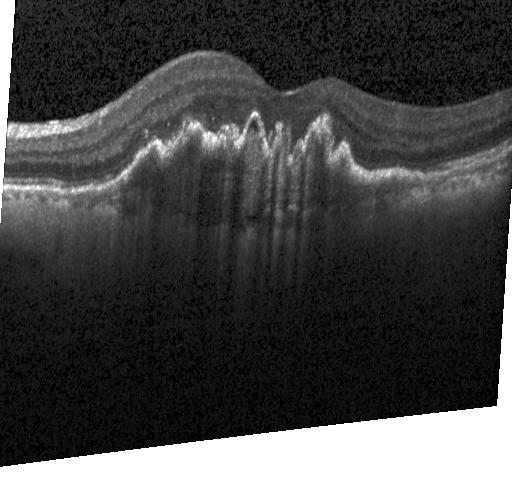

Impression: a choroidal neovascular membrane.